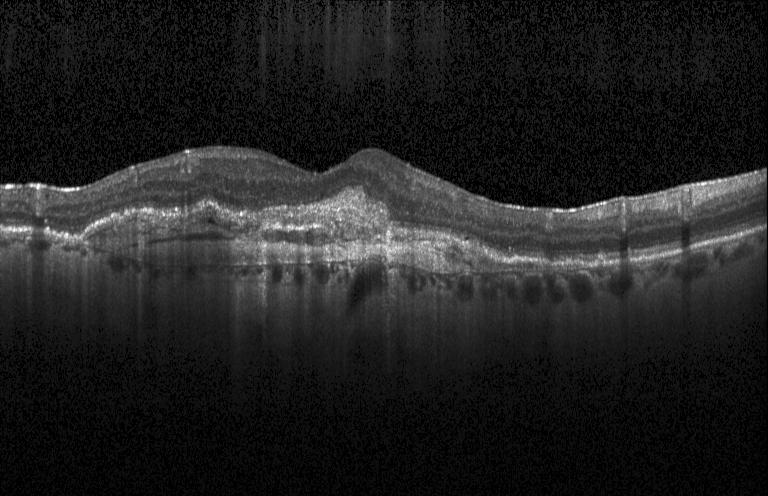
Macular OCT demonstrating a choroidal neovascular membrane.